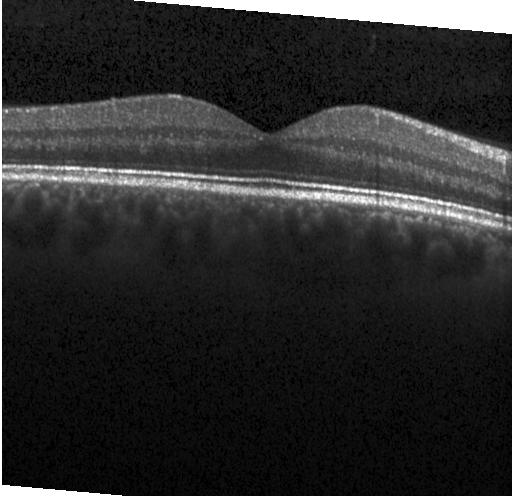 Dx: no CNV, DME, or drusen.